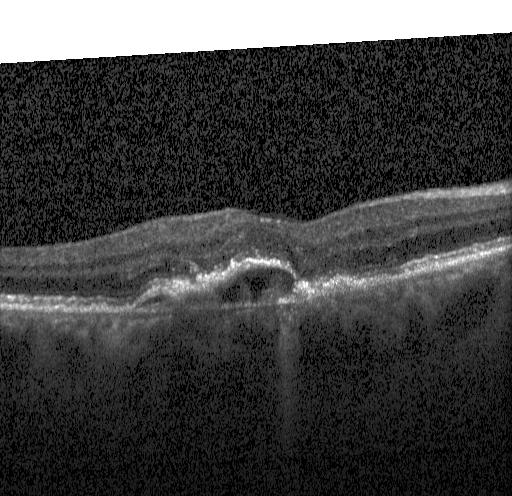
Retinal OCT cross-section showing choroidal neovascularization (CNV).